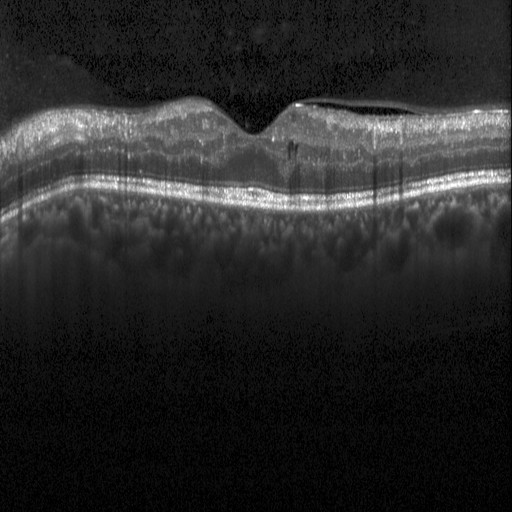

Macular OCT: DME.